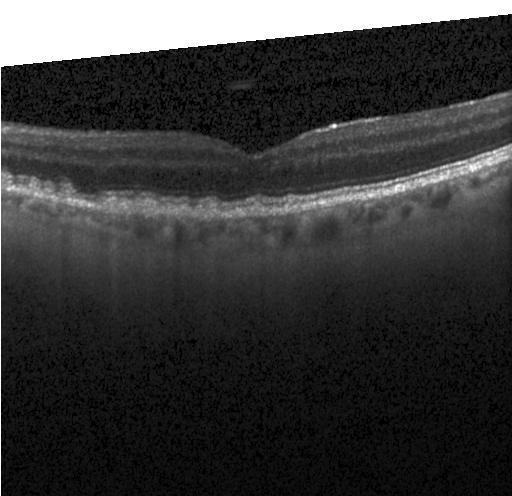
Finding: drusen.